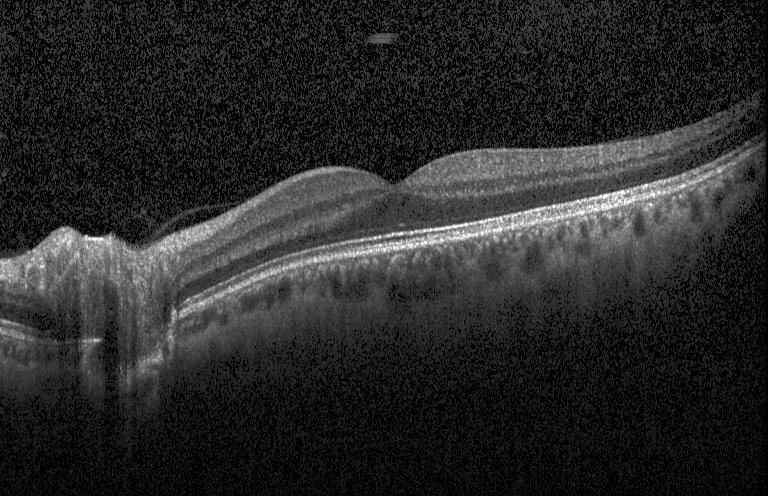

Neither choroidal neovascularization, diabetic macular edema, nor drusen.